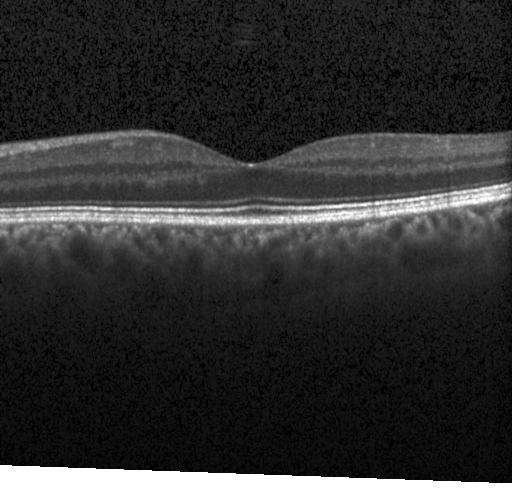

Retinal OCT cross-section showing no choroidal neovascularization, no diabetic macular edema, and no drusen.